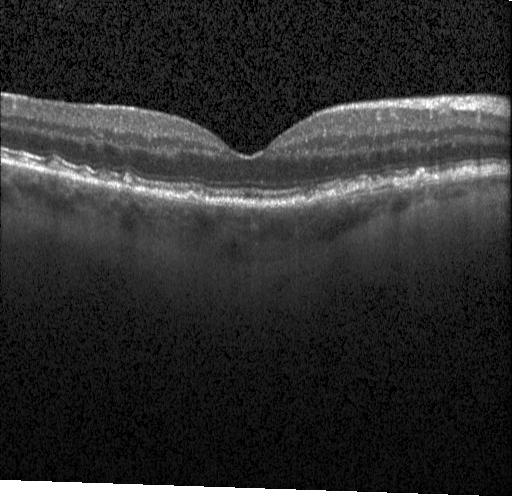

Retinal OCT B-scan
This B-scan demonstrates sub-RPE drusenoid deposits.